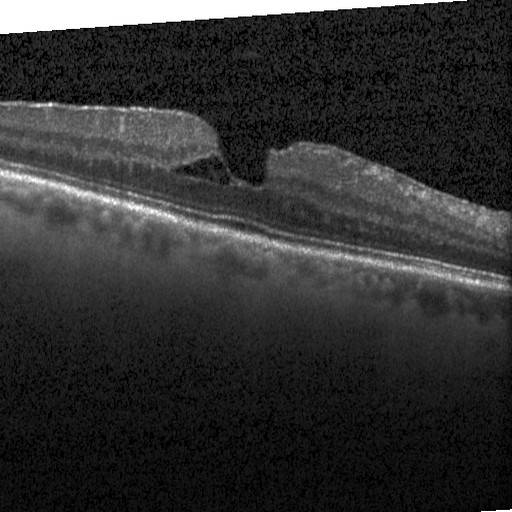 Macular OCT: DME.